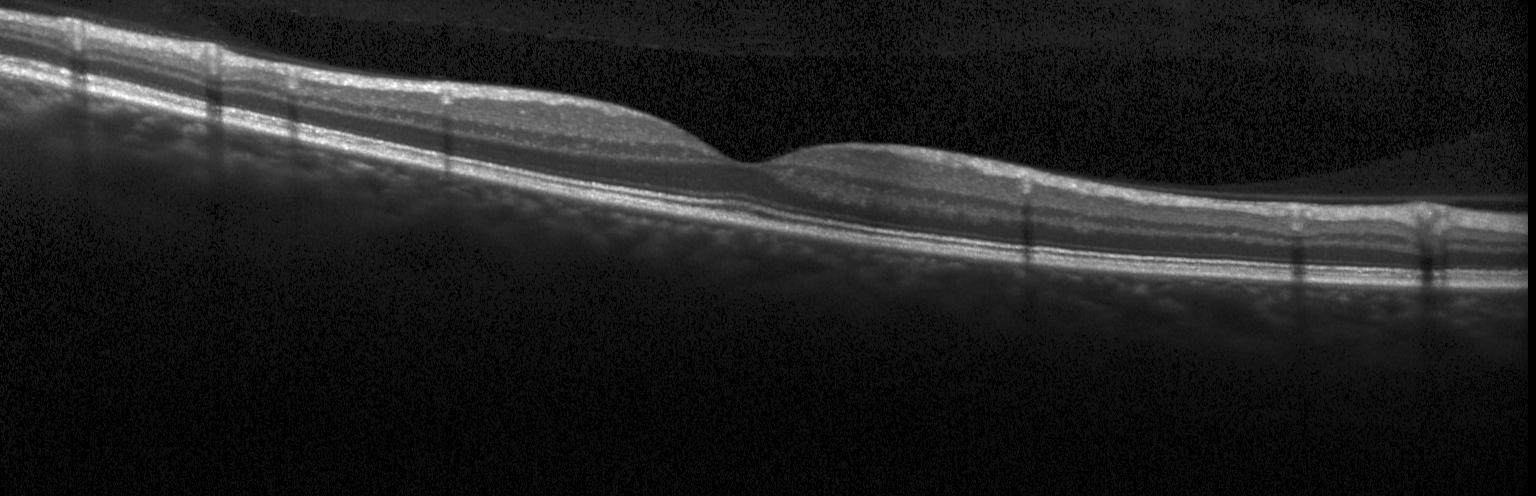 Impression: neither choroidal neovascularization, diabetic macular edema, nor drusen.